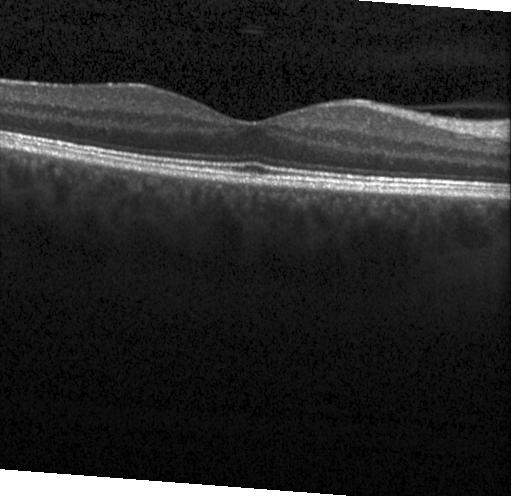
Finding: neither choroidal neovascularization, diabetic macular edema, nor drusen.